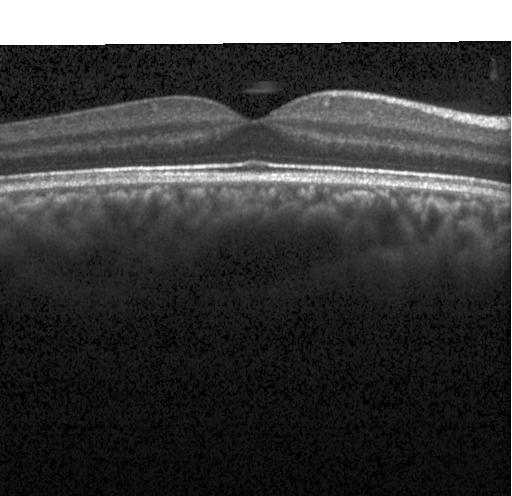
OCT B-scan; SD-OCT — Diagnosis: no evidence of choroidal neovascularization, diabetic macular edema, or drusen.